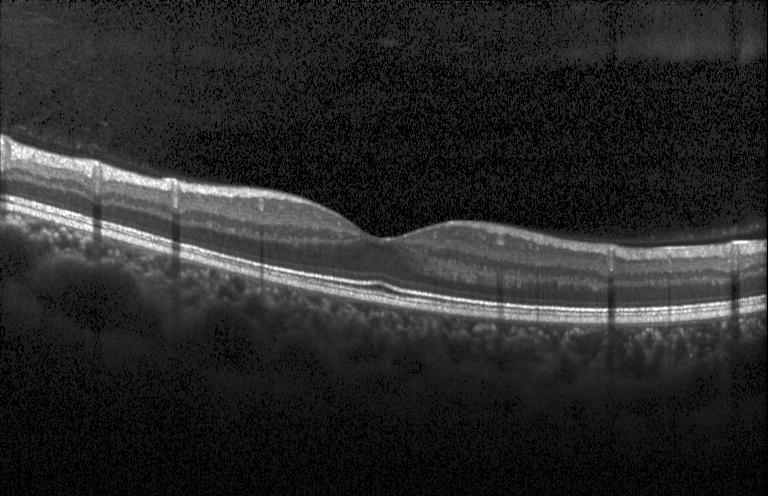 Impression: no choroidal neovascularization, no diabetic macular edema, and no drusen.